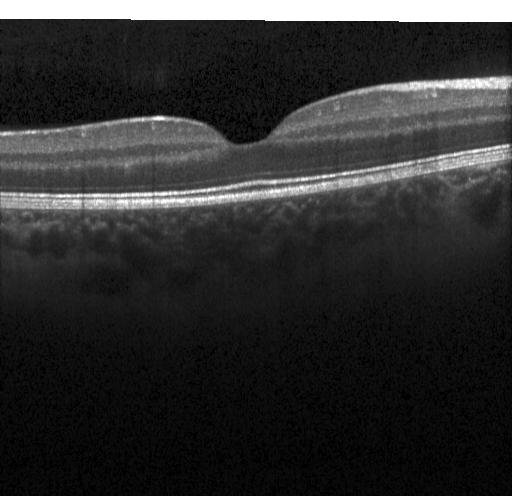 Heidelberg Spectralis OCT system; retinal OCT B-scan.
Impression: no CNV, DME, or drusen.